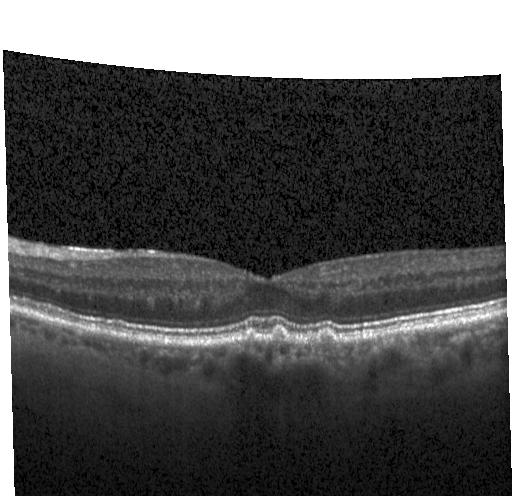
Drusen.